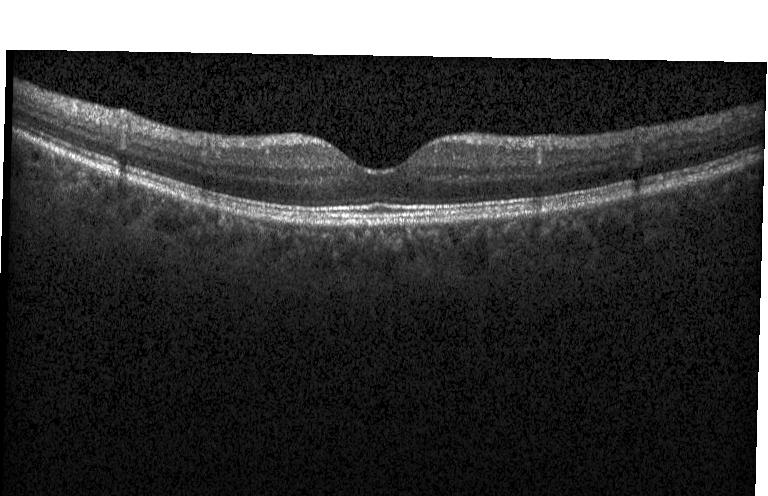
Macular scan · retinal OCT B-scan · SD-OCT · Heidelberg Spectralis.
Diagnosis: no CNV, no DME, and no drusen.